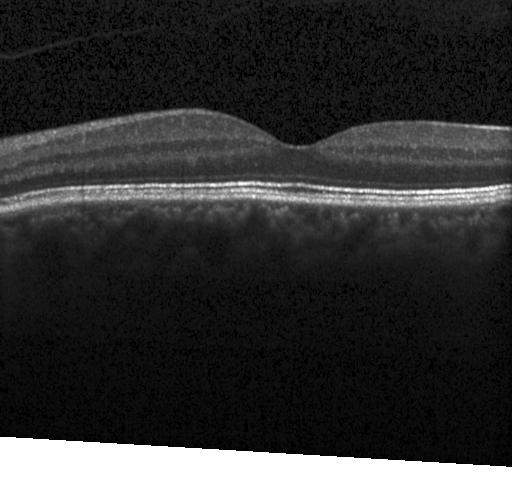

Spectral-domain optical coherence tomography, optical coherence tomography B-scan.
Assessment: no choroidal neovascularization, diabetic macular edema, or drusen.